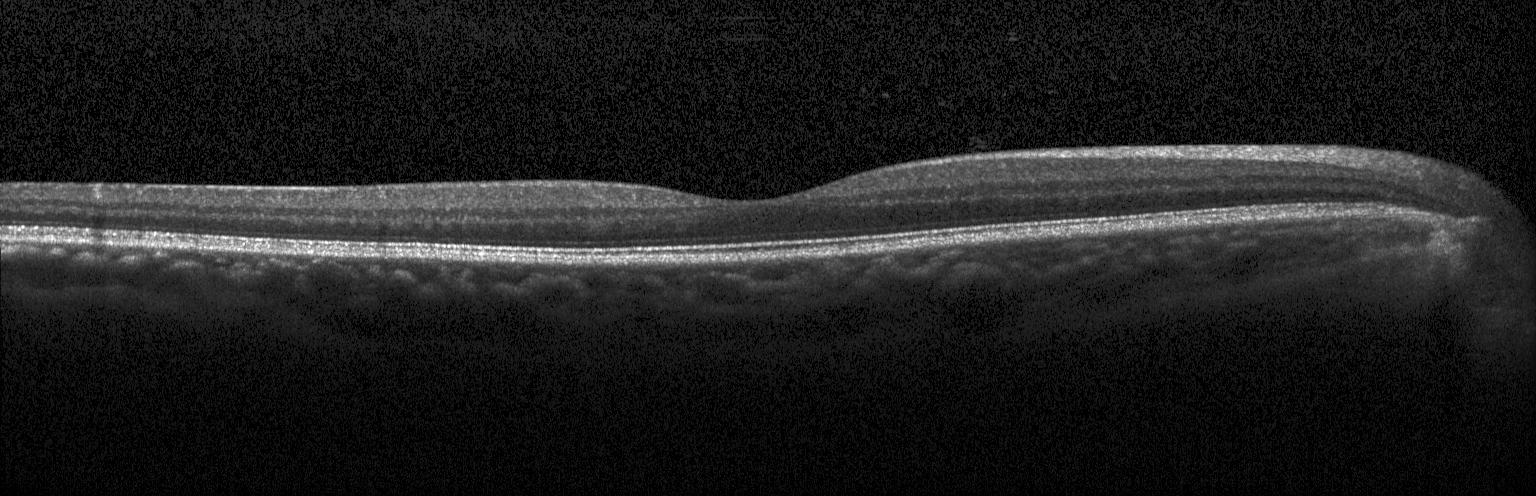 No evidence of choroidal neovascularization, diabetic macular edema, or drusen.